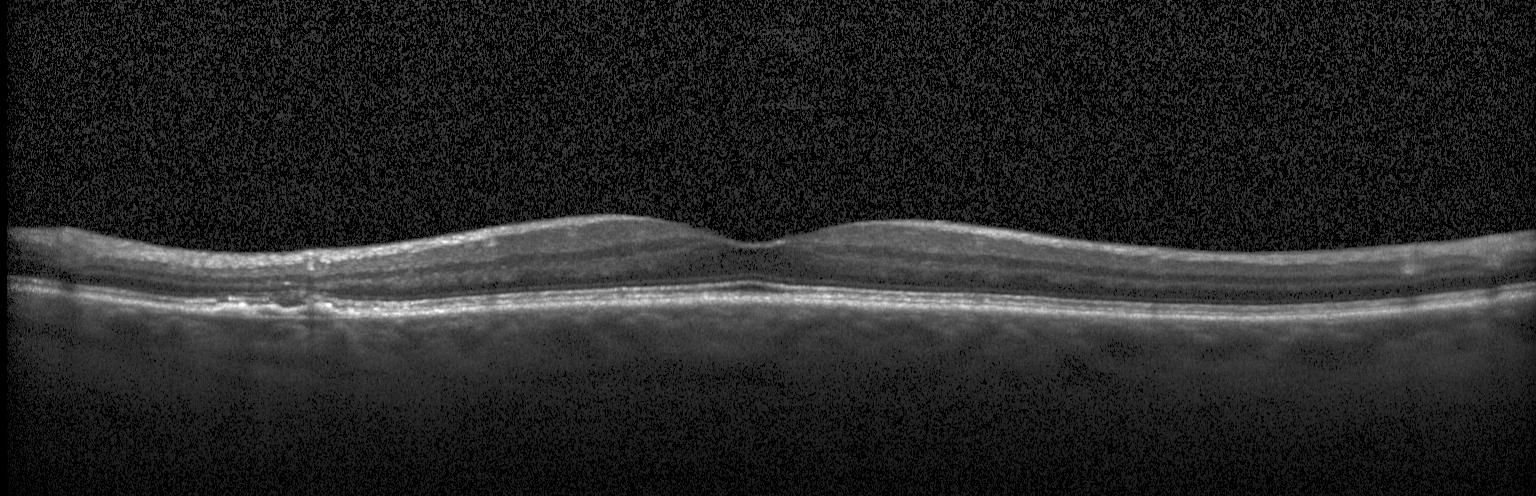
Dx: choroidal neovascularization.